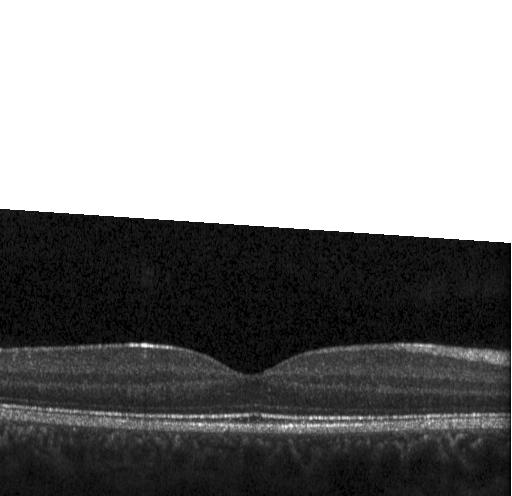

Macular scan; retinal OCT cross-section; spectral-domain optical coherence tomography; Heidelberg Spectralis — Finding: neither choroidal neovascularization, diabetic macular edema, nor drusen.